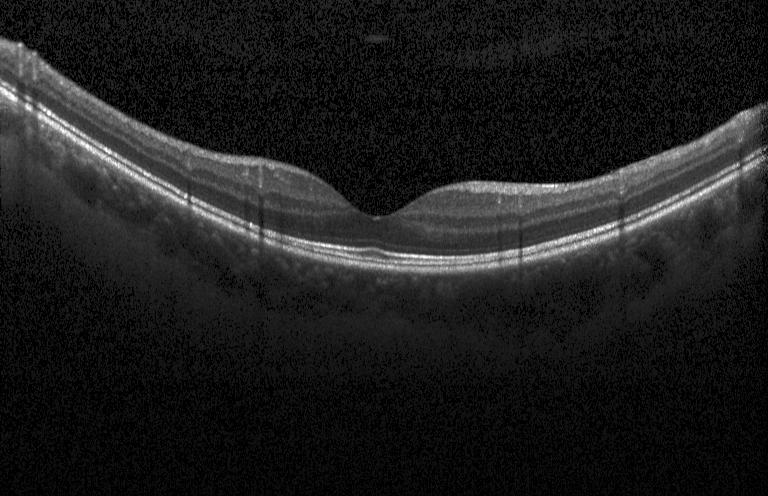
Diagnosis: no choroidal neovascularization, no diabetic macular edema, and no drusen.